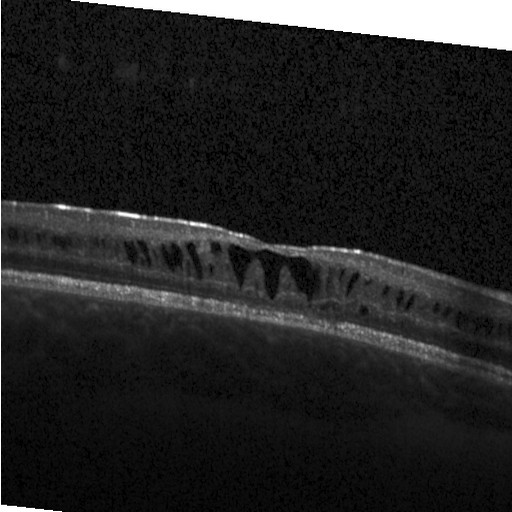

Spectral-domain OCT; retinal OCT cross-section; Heidelberg Spectralis. Diabetic macular edema (DME).